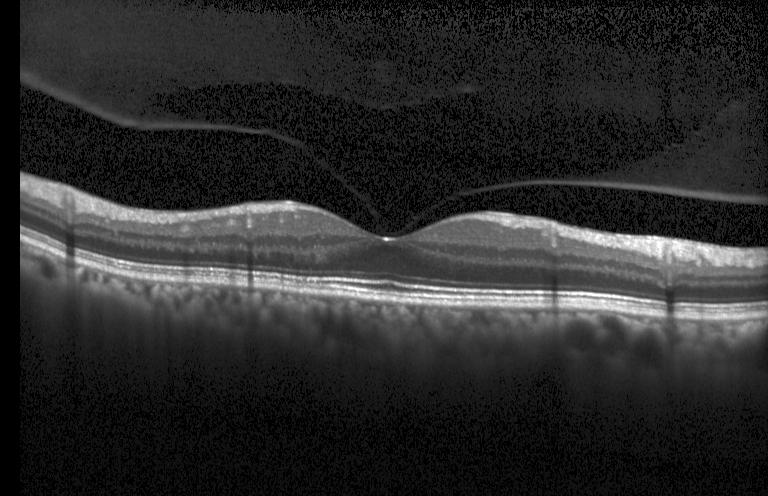 Diagnosis: no evidence of choroidal neovascularization, diabetic macular edema, or drusen.